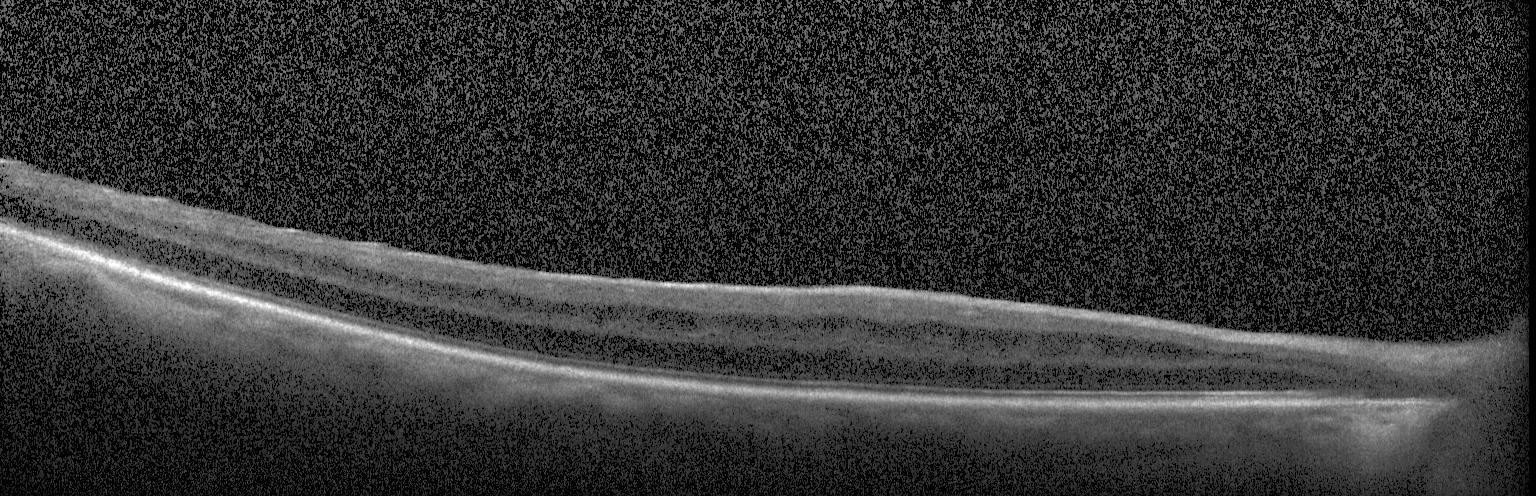
Optical coherence tomography scan. The scan shows diabetic macular edema.